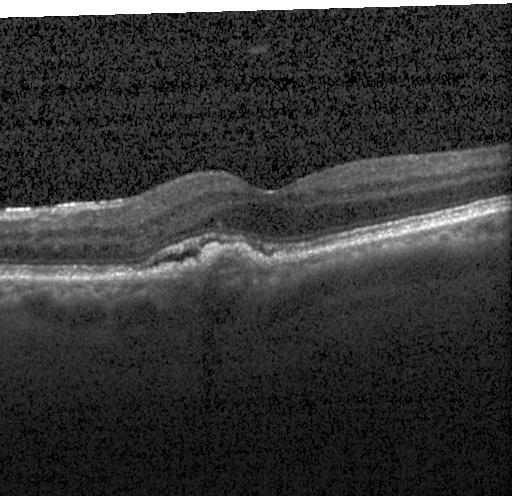
Macular OCT: choroidal neovascularization.